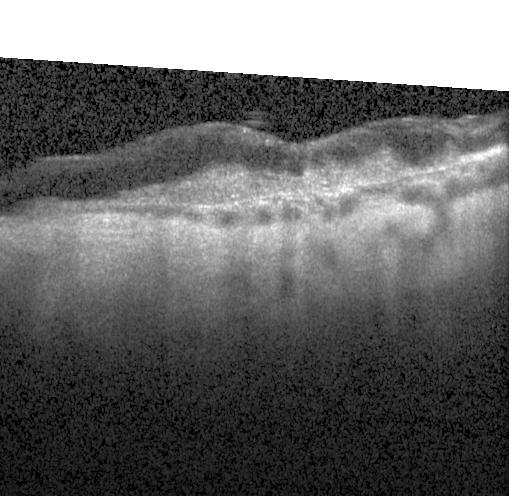 Heidelberg Spectralis · OCT line scan · centered on the fovea · spectral-domain optical coherence tomography
Impression: CNV.